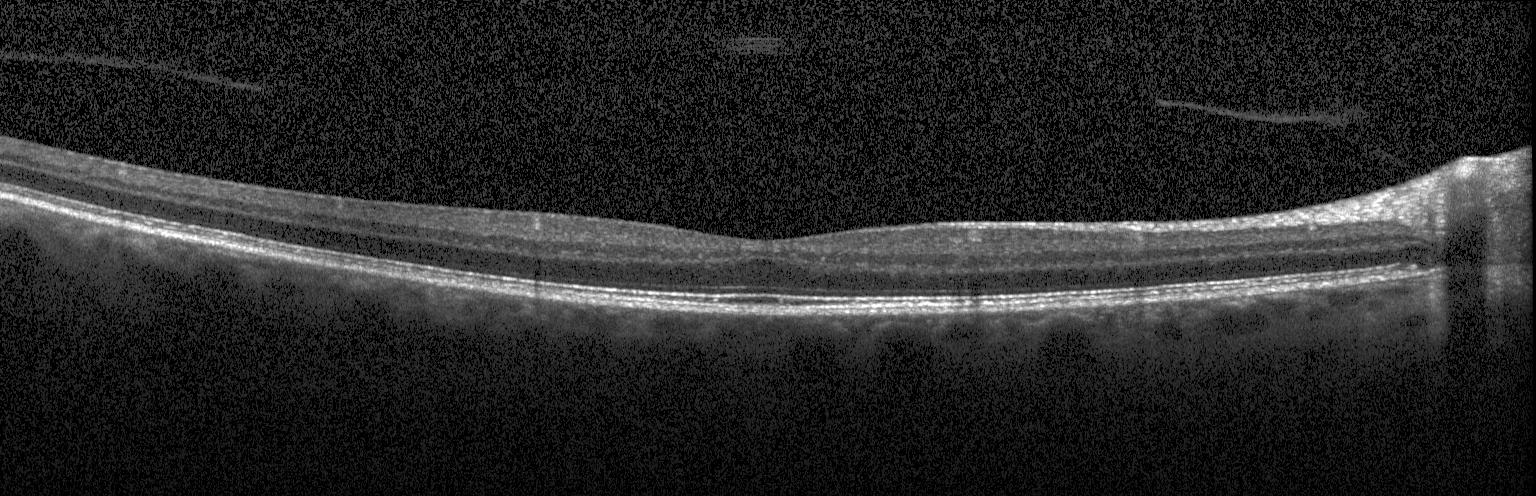

SD-OCT. Retinal OCT cross-section. Centered on the fovea.
No choroidal neovascularization, diabetic macular edema, or drusen.